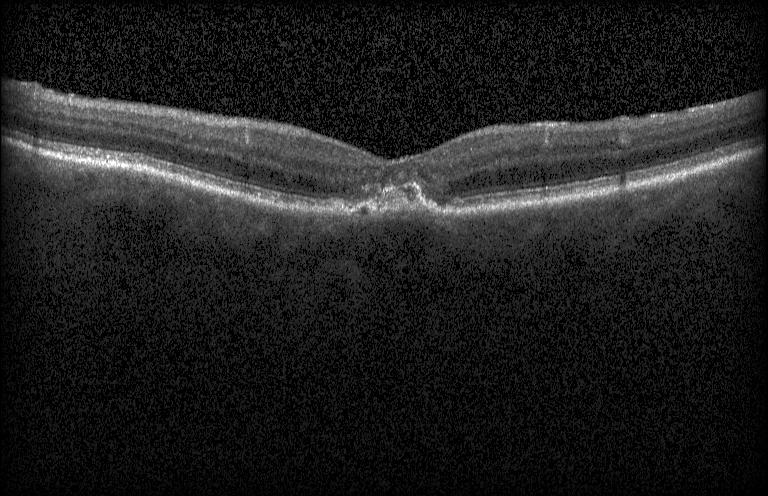

Heidelberg Spectralis. Spectral-domain OCT. Fovea-centered. OCT line scan. The scan shows a choroidal neovascular membrane.